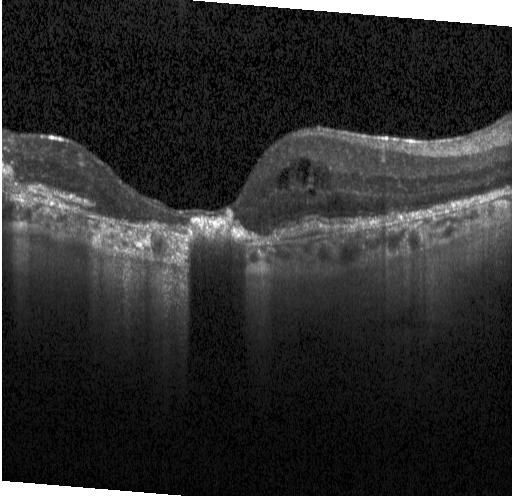

Diagnosis: CNV.